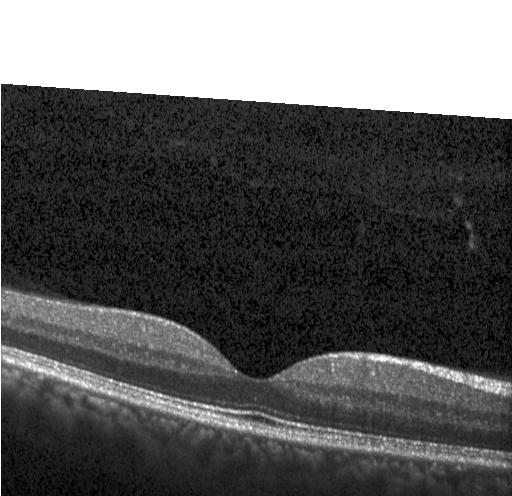 Spectral-domain OCT B-scan: no CNV, DME, or drusen.